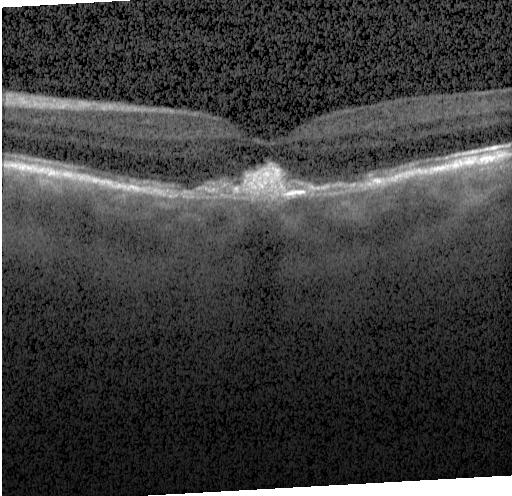 OCT line scan
Finding: choroidal neovascularization.